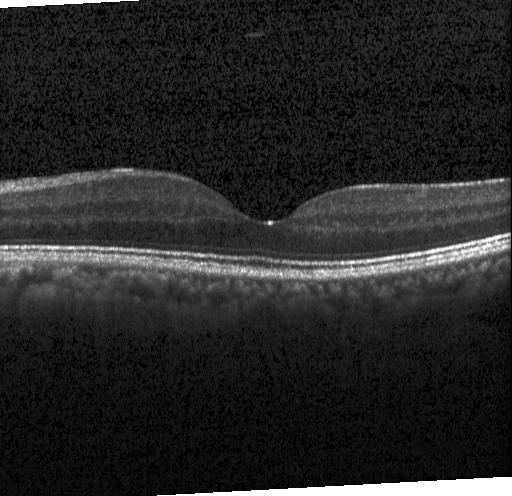
Spectral-domain optical coherence tomography. Macular scan. OCT B-scan. Acquired on a Heidelberg Spectralis — This B-scan demonstrates no evidence of choroidal neovascularization, diabetic macular edema, or drusen.